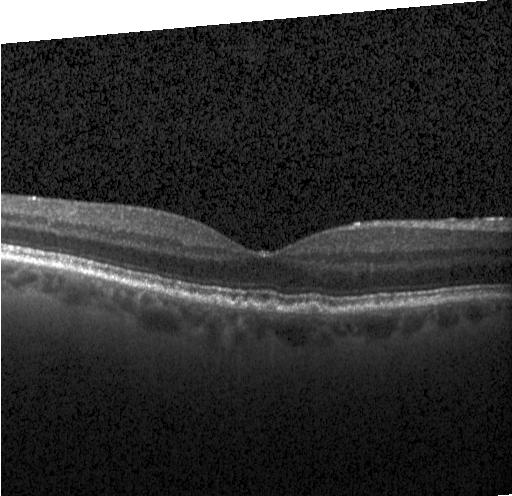
Assessment: sub-RPE drusenoid deposits.